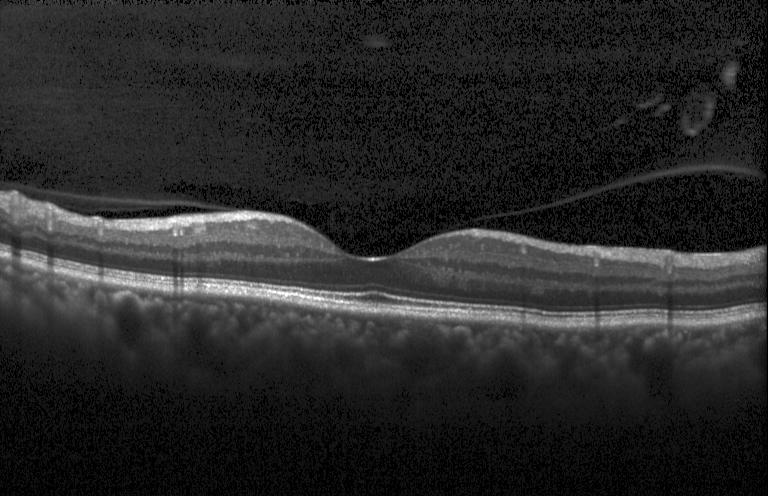
Impression: no evidence of choroidal neovascularization, diabetic macular edema, or drusen.